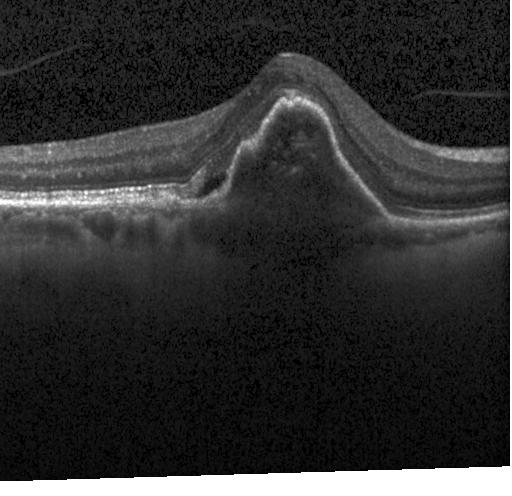

Heidelberg Spectralis OCT system · horizontal scan through the fovea · retinal OCT cross-section · SD-OCT.
Impression: a choroidal neovascular membrane.